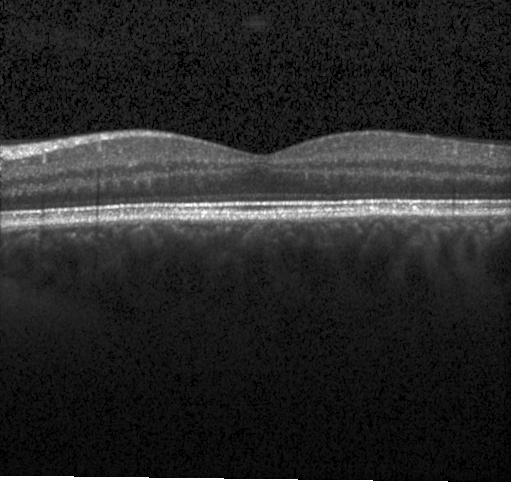

OCT line scan. This B-scan demonstrates no choroidal neovascularization, no diabetic macular edema, and no drusen.